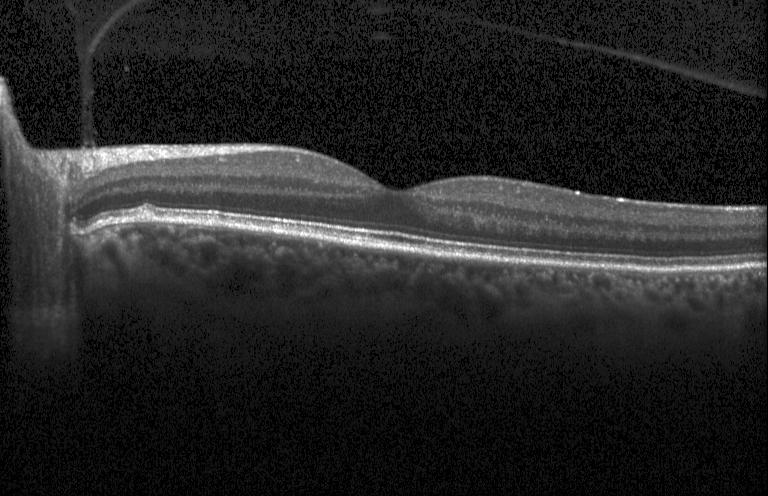
Diagnosis: multiple drusen.